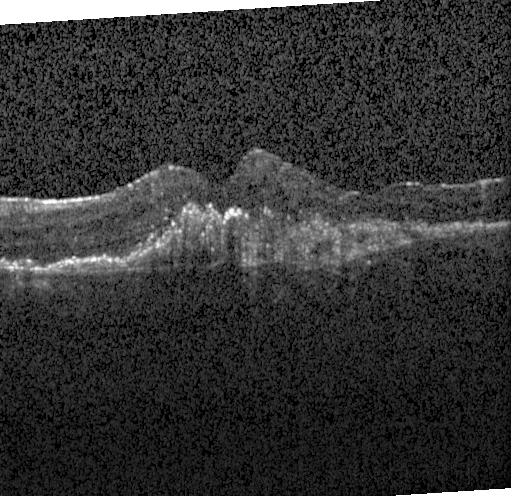 OCT line scan; macular scan; spectral-domain OCT — Dx: a choroidal neovascular membrane.